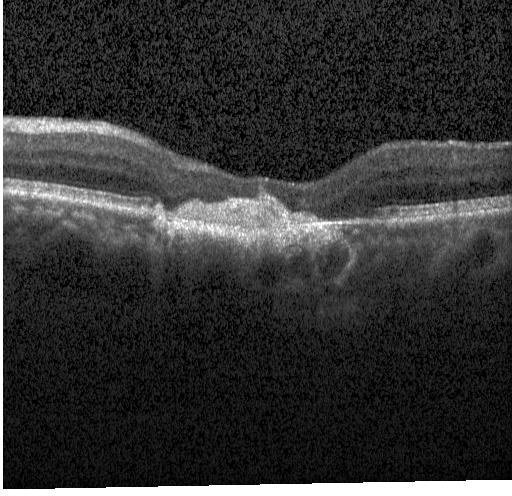 OCT finding: a choroidal neovascular membrane.